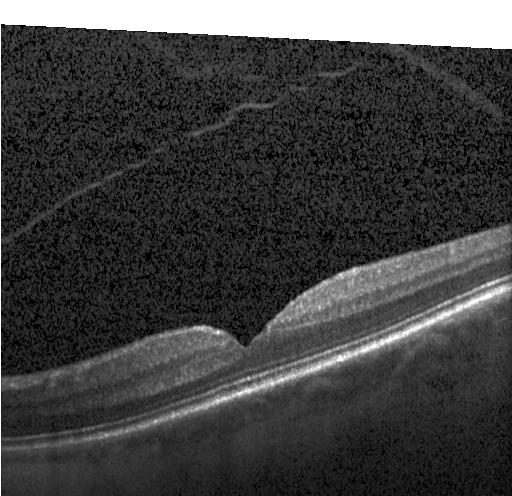
Retinal OCT B-scan — Impression: neither CNV, DME, nor drusen.